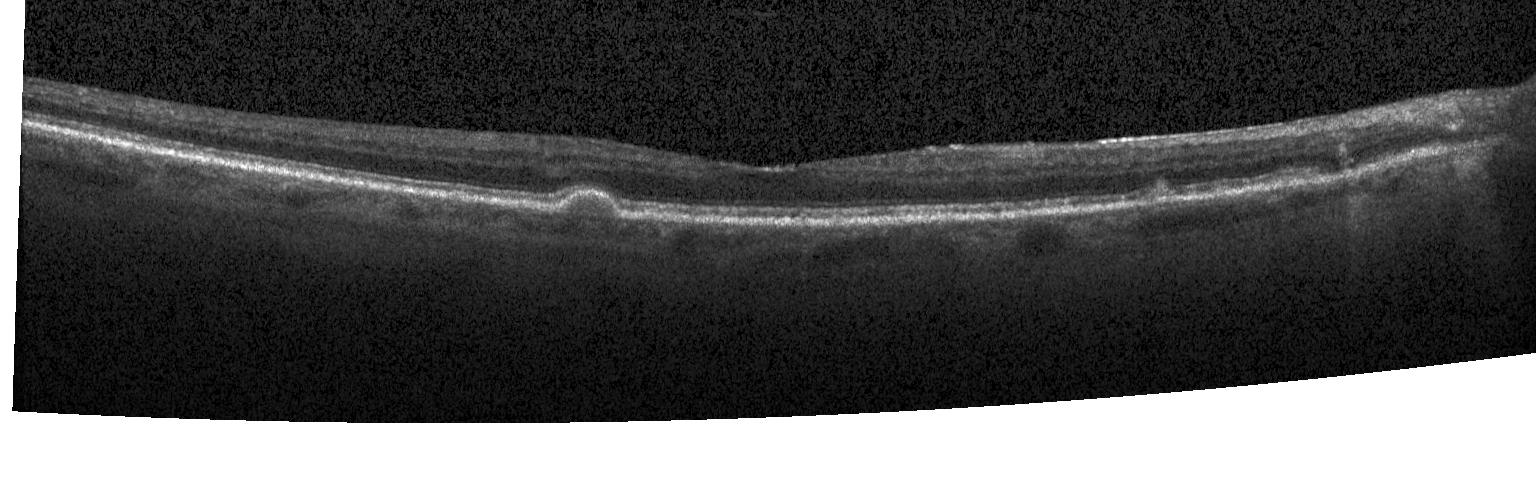

Impression: multiple drusen.